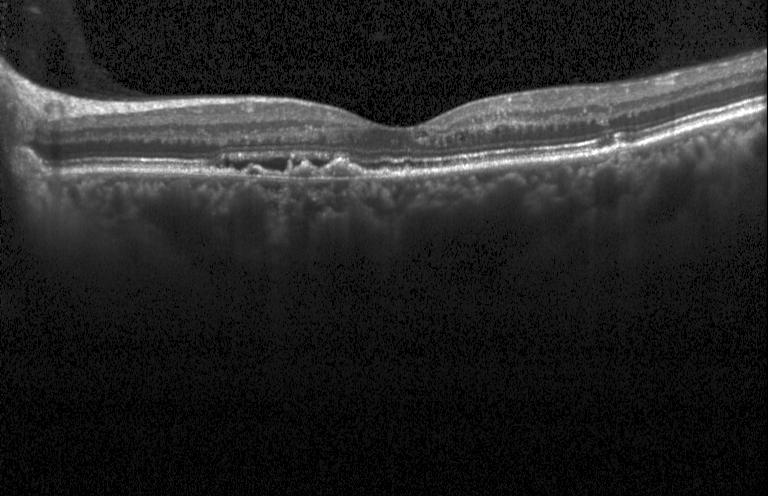

Macular scan. Heidelberg Spectralis. Spectral-domain OCT. OCT line scan.
This B-scan demonstrates CNV.